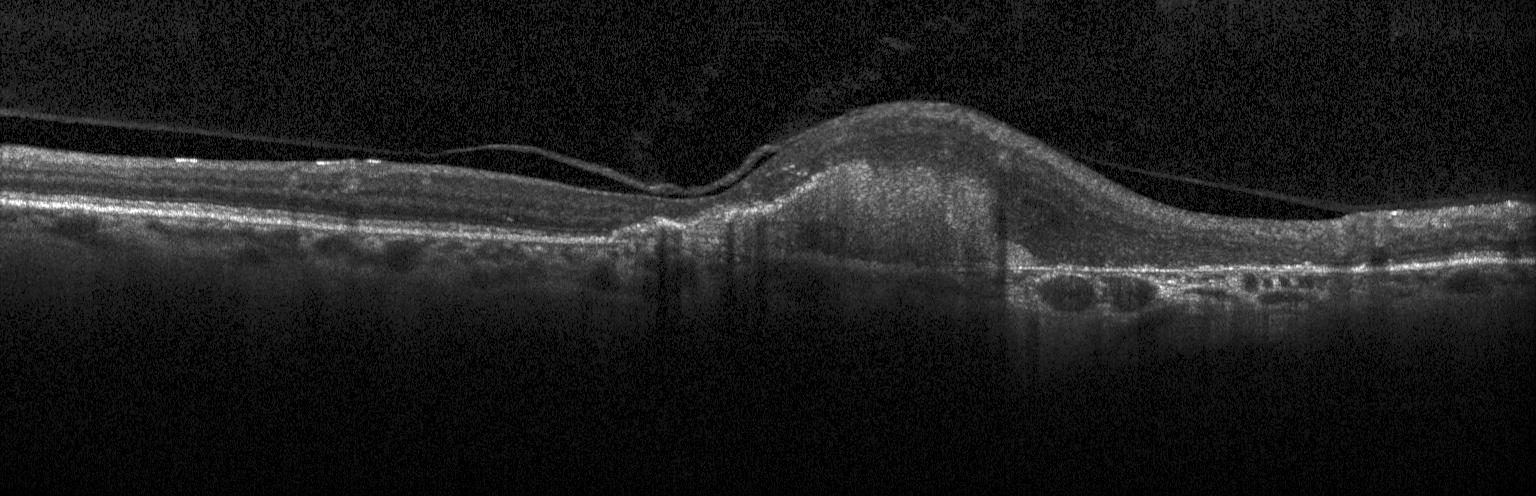
Spectral-domain optical coherence tomography, retinal OCT cross-section. CNV.